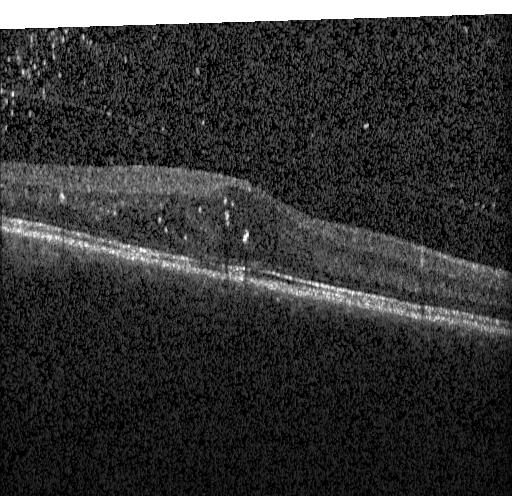 OCT finding: diabetic macular edema.